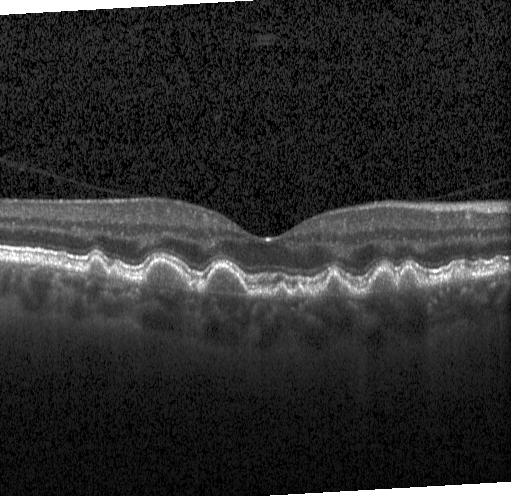

OCT line scan. Macular scan. Instrument: Heidelberg Spectralis. Spectral-domain OCT. Diagnosis: multiple drusen.